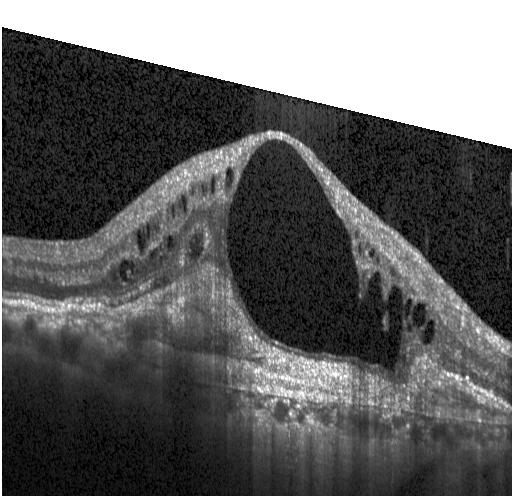
Finding: a choroidal neovascular membrane.